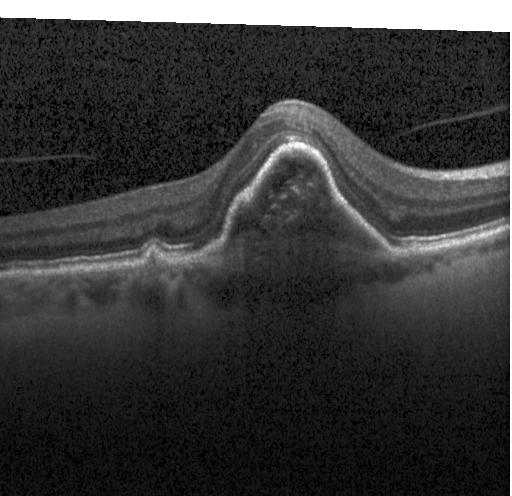

Fovea-centered, optical coherence tomography scan, SD-OCT.
A choroidal neovascular membrane.